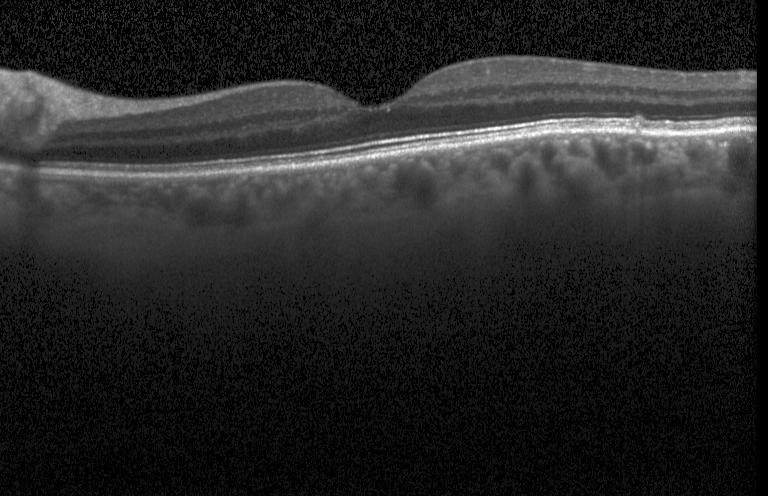

Optical coherence tomography B-scan. Impression: drusen.